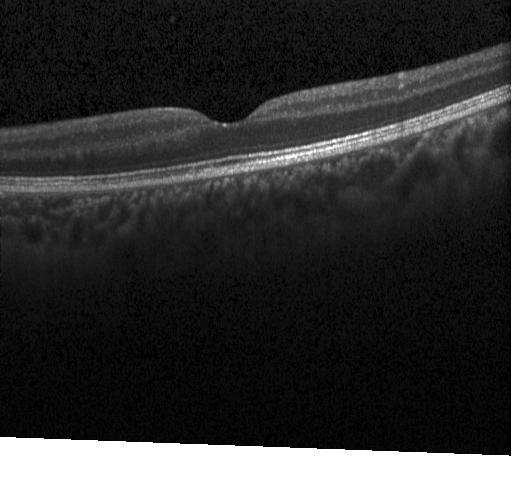
Optical coherence tomography B-scan — Finding: no choroidal neovascularization, diabetic macular edema, or drusen.